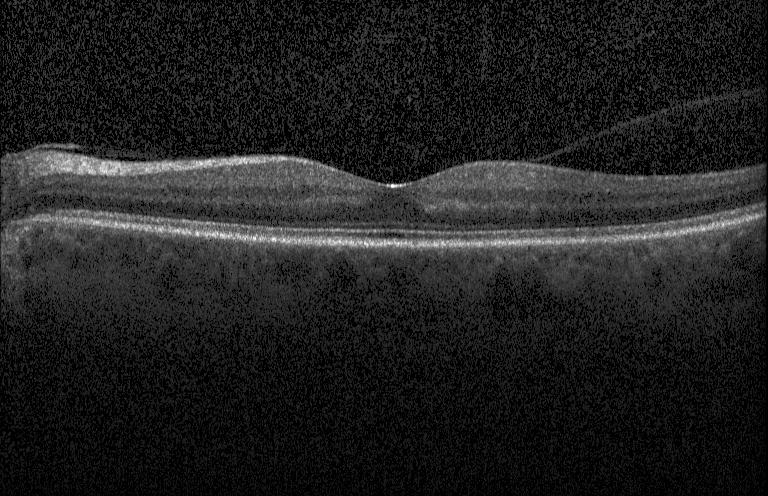 Optical coherence tomography B-scan; SD-OCT; acquired on a Heidelberg Spectralis. Macular OCT: neither choroidal neovascularization, diabetic macular edema, nor drusen.